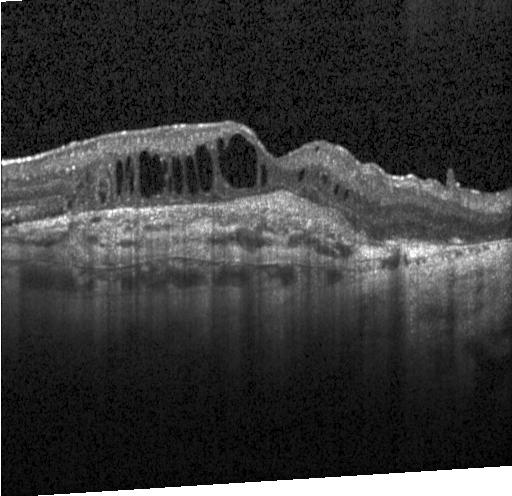 Macular OCT demonstrating CNV.